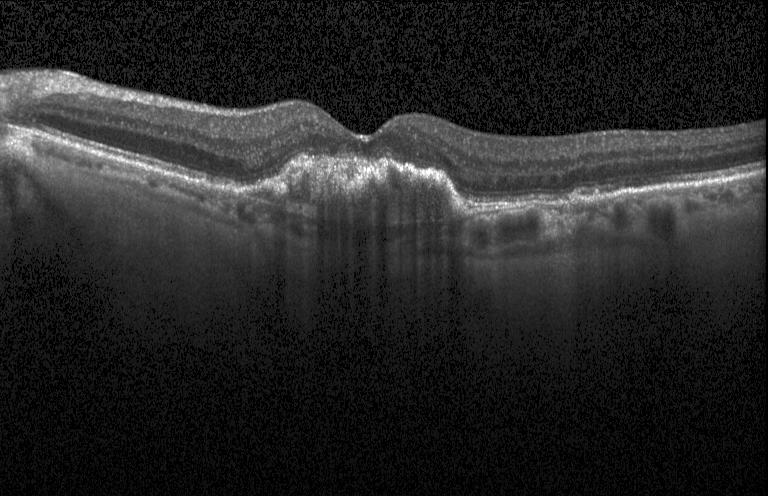
Spectral-domain OCT · retinal OCT B-scan · Heidelberg Spectralis OCT system
Diagnosis: choroidal neovascularization.